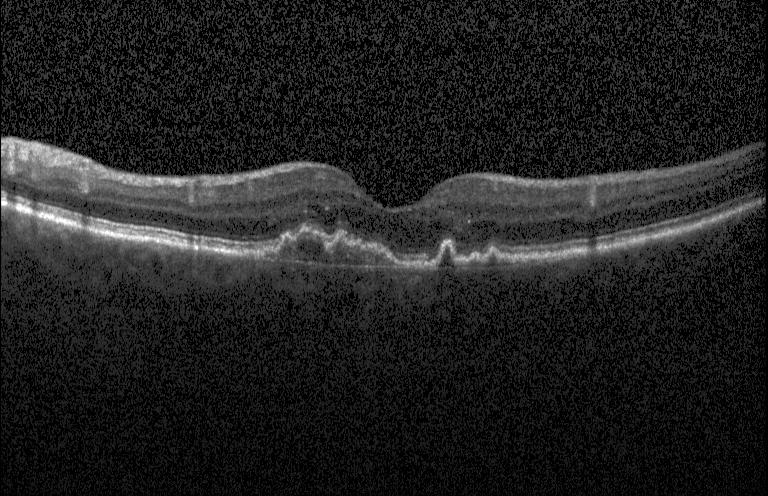

Acquired on a Heidelberg Spectralis, SD-OCT, centered on the fovea, OCT B-scan — A choroidal neovascular membrane.